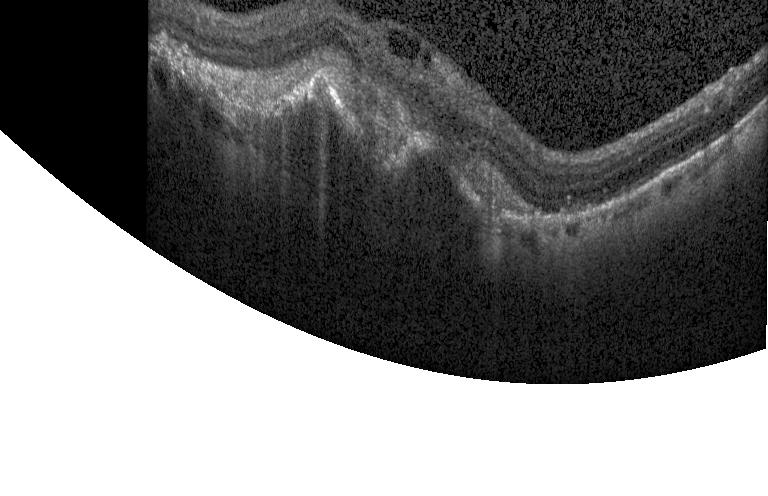

Dx: a choroidal neovascular membrane.